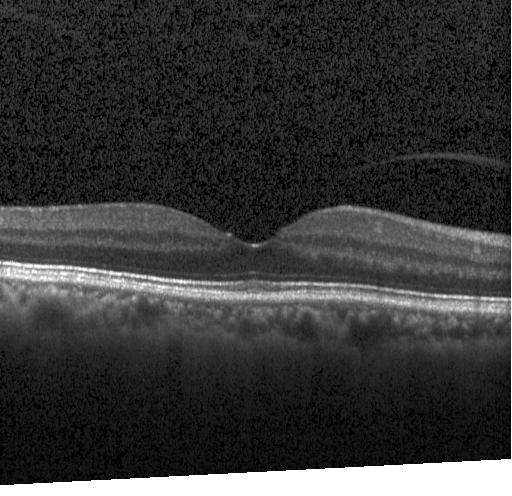 Centered on the fovea · spectral-domain optical coherence tomography · optical coherence tomography scan · Heidelberg Spectralis — No evidence of choroidal neovascularization, diabetic macular edema, or drusen.